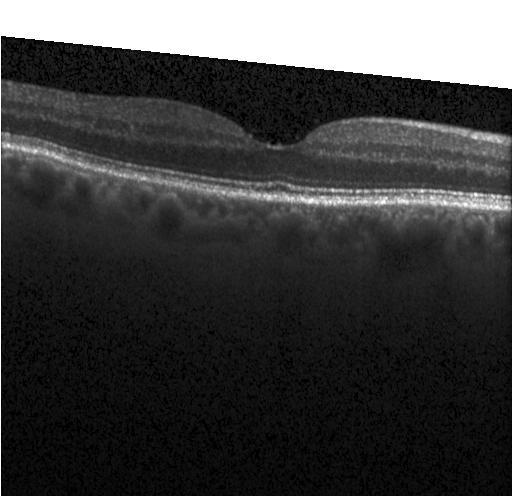
Optical coherence tomography B-scan — Impression: no choroidal neovascularization, no diabetic macular edema, and no drusen.